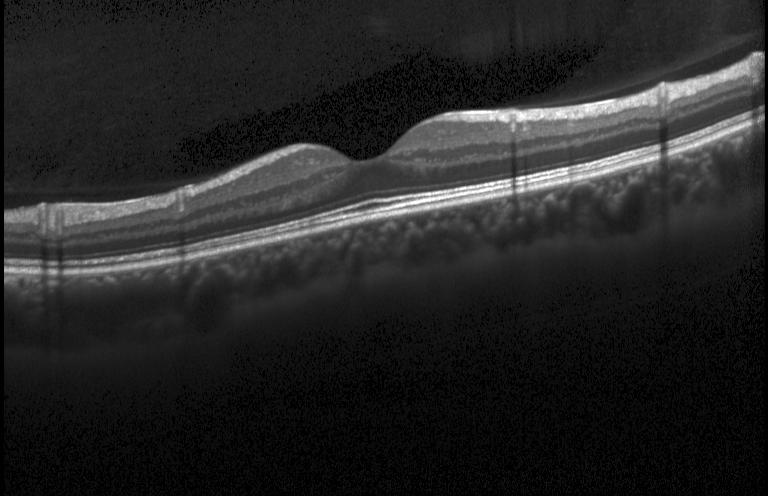
SD-OCT, Heidelberg Spectralis OCT system, OCT B-scan, fovea-centered. Dx: no CNV, no DME, and no drusen.